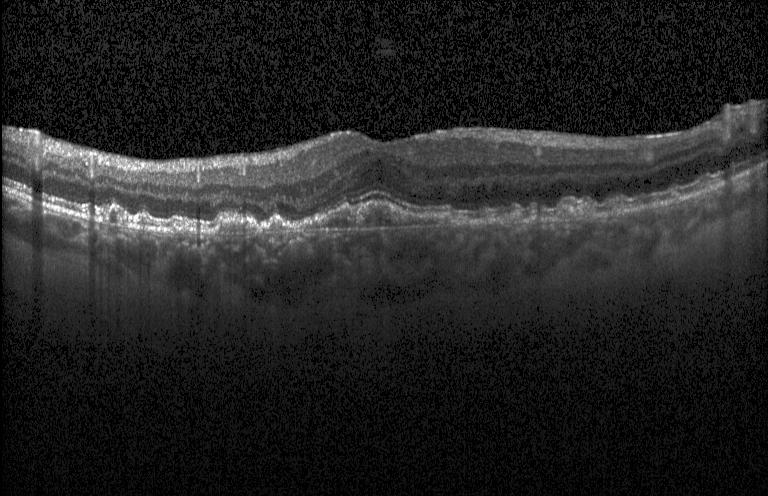
Heidelberg Spectralis. Centered on the fovea. Retinal OCT B-scan. This B-scan demonstrates CNV.